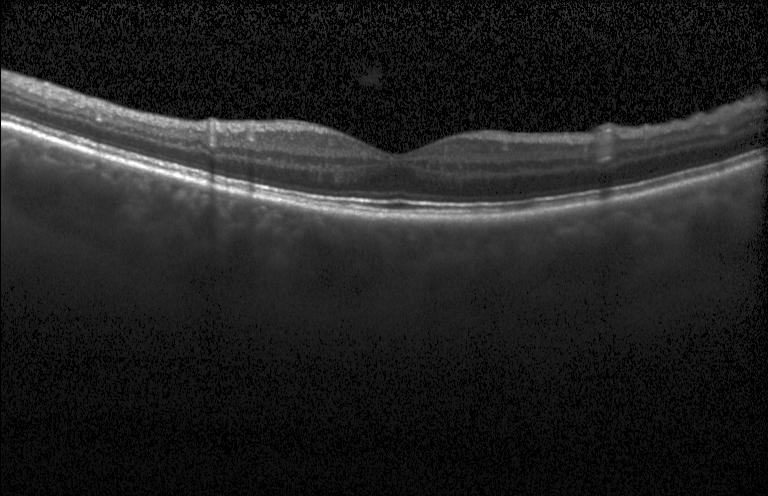
Macular scan. SD-OCT. Retinal OCT B-scan. Acquired on a Heidelberg Spectralis
The scan shows no choroidal neovascularization, no diabetic macular edema, and no drusen.